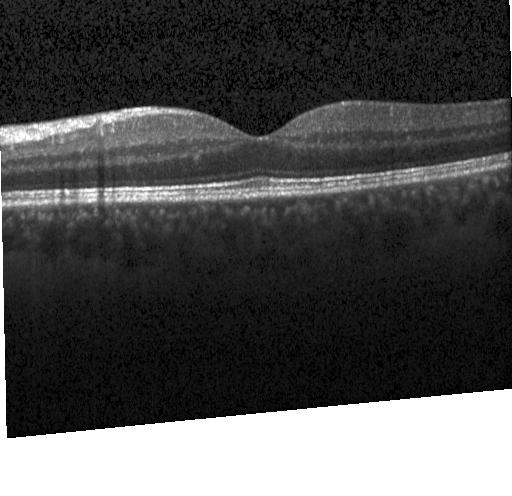
Retinal OCT B-scan · Heidelberg Spectralis — Macular OCT: neither choroidal neovascularization, diabetic macular edema, nor drusen.